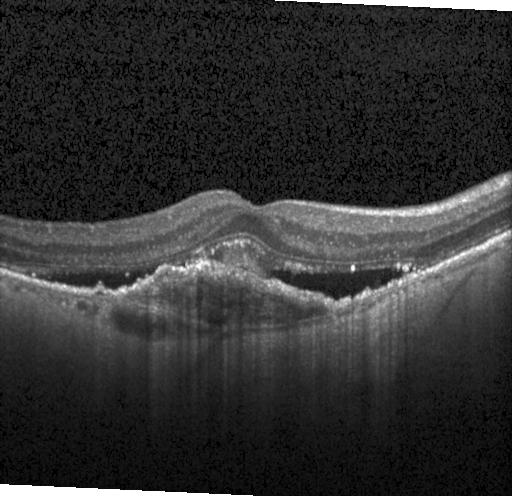

Assessment: choroidal neovascularization (CNV).